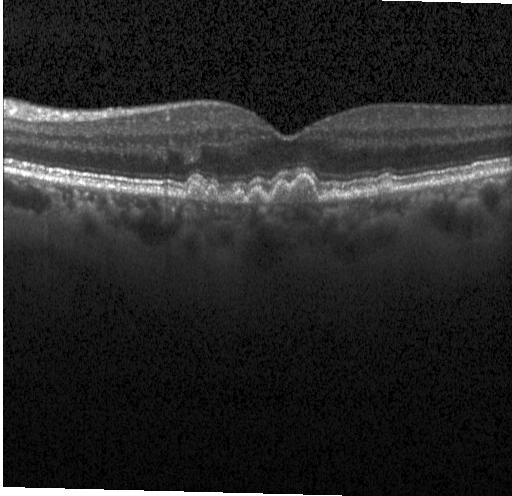
Assessment: sub-RPE drusenoid deposits.